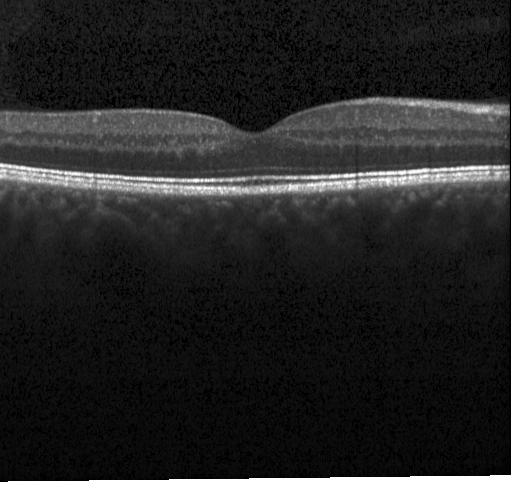
Optical coherence tomography B-scan · Heidelberg Spectralis. Diagnosis: no CNV, no DME, and no drusen.